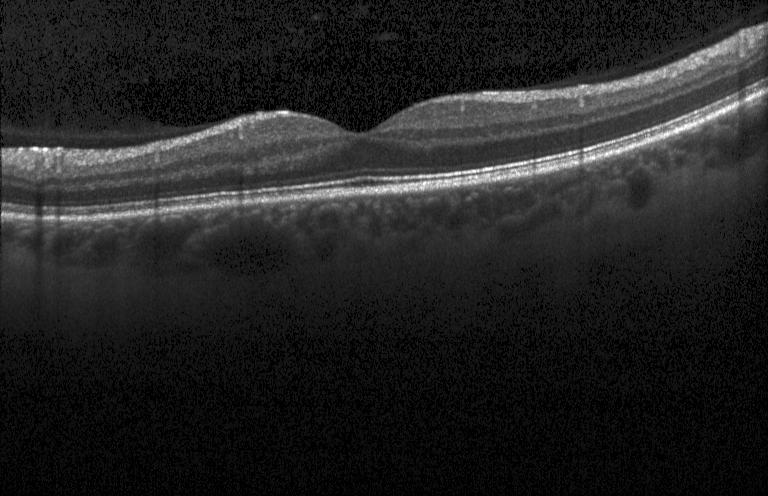 OCT B-scan showing no evidence of CNV, DME, or drusen.